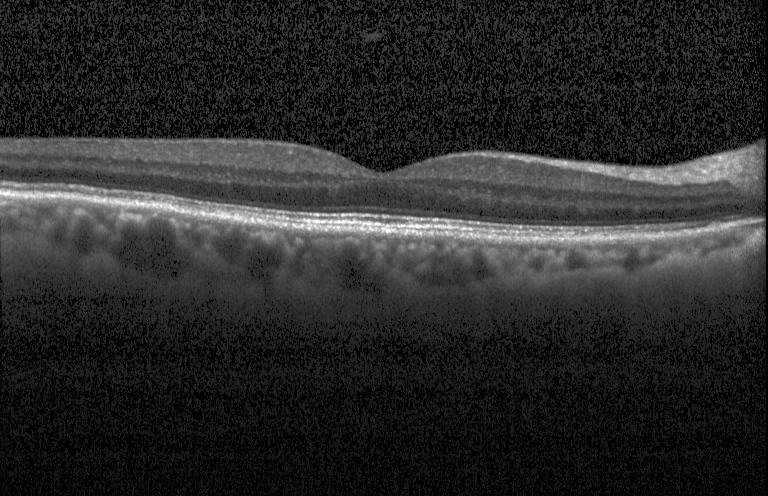

Centered on the fovea · SD-OCT · optical coherence tomography B-scan · Heidelberg Spectralis OCT system — Assessment: neither choroidal neovascularization, diabetic macular edema, nor drusen.